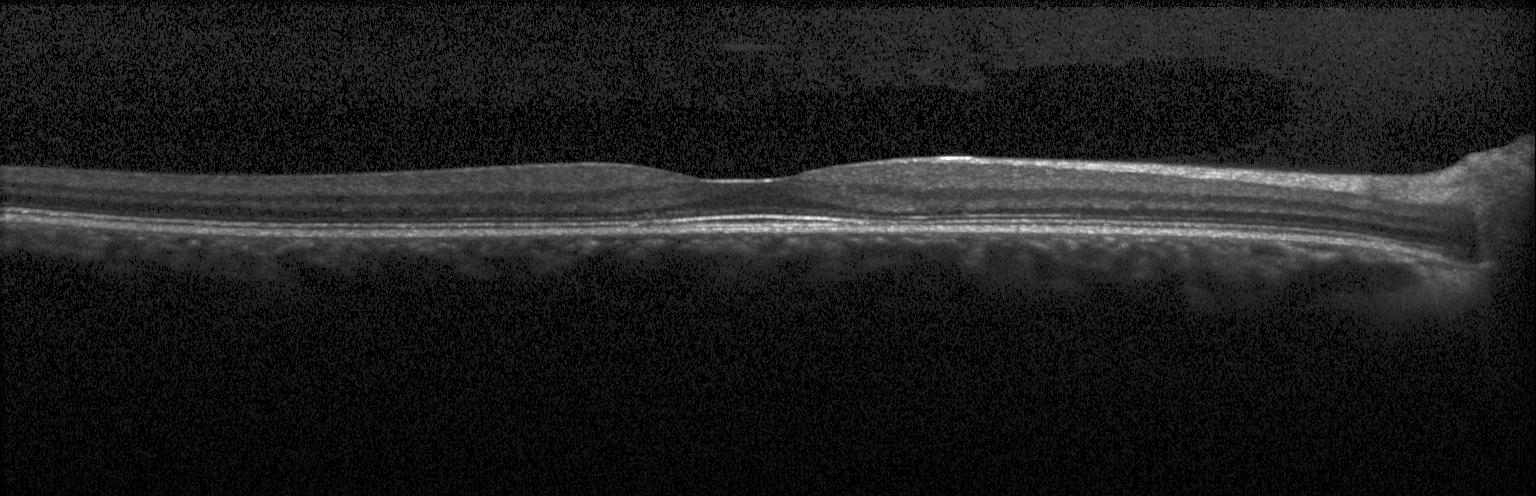
Macular OCT: no choroidal neovascularization, no diabetic macular edema, and no drusen.